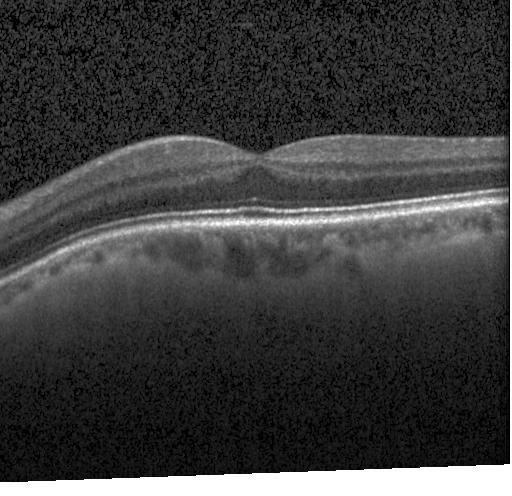
Optical coherence tomography scan, acquired on a Heidelberg Spectralis, centered on the fovea, spectral-domain optical coherence tomography
No choroidal neovascularization, diabetic macular edema, or drusen.